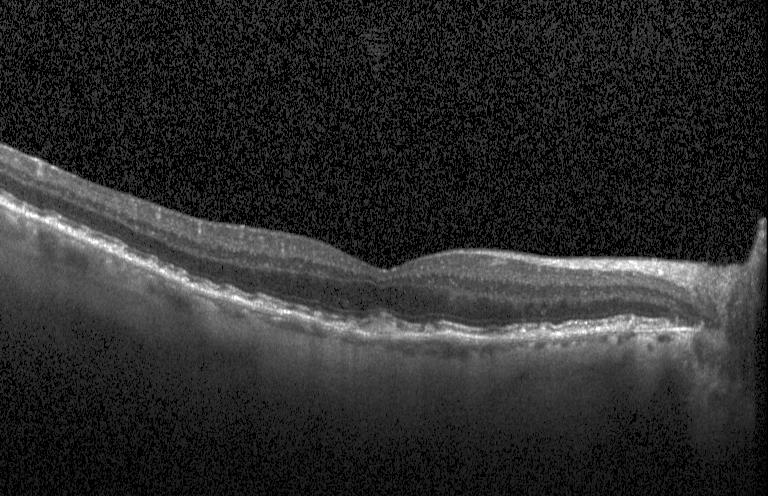
Retinal OCT B-scan; spectral-domain optical coherence tomography. Finding: drusen.